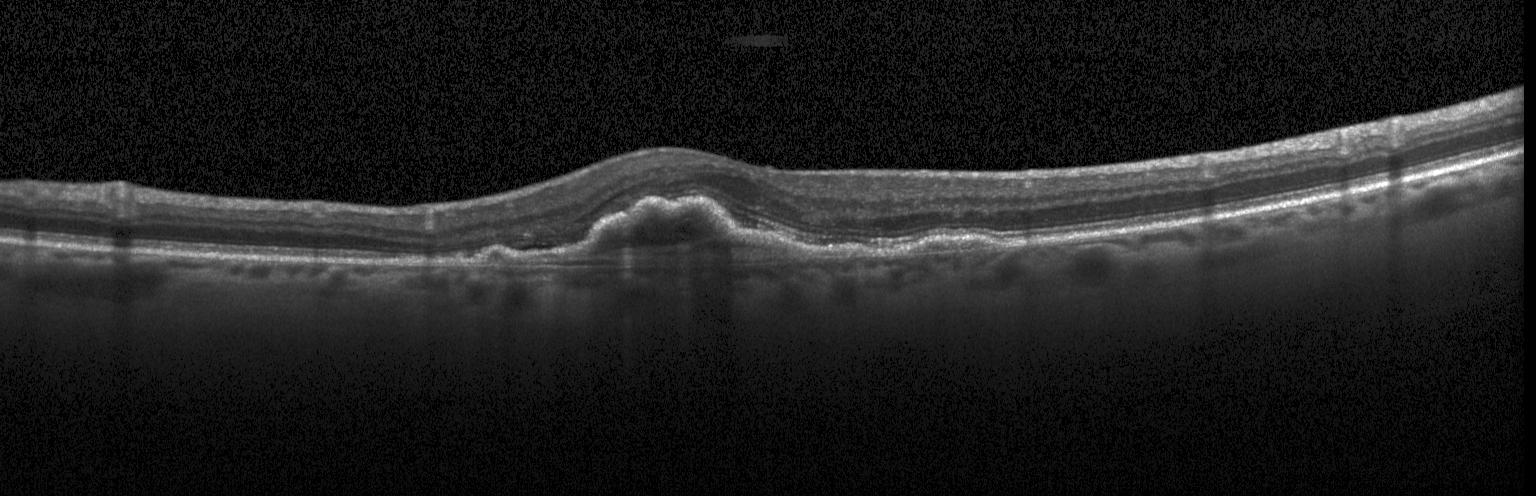 Retinal OCT cross-section showing choroidal neovascularization.